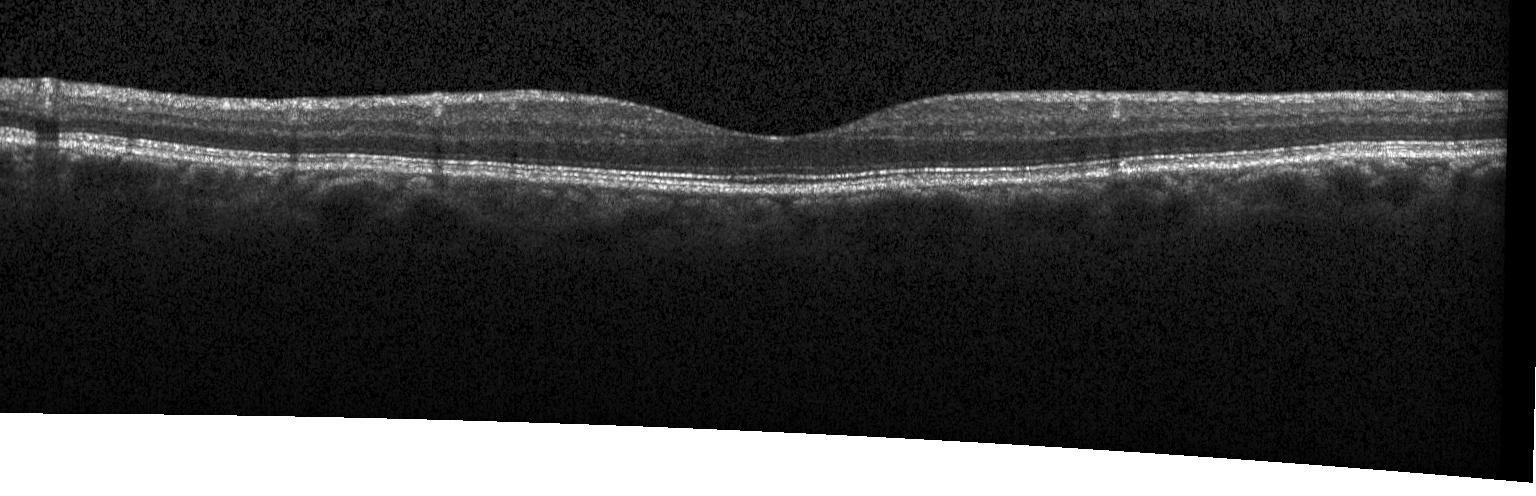

Finding: no choroidal neovascularization, no diabetic macular edema, and no drusen.